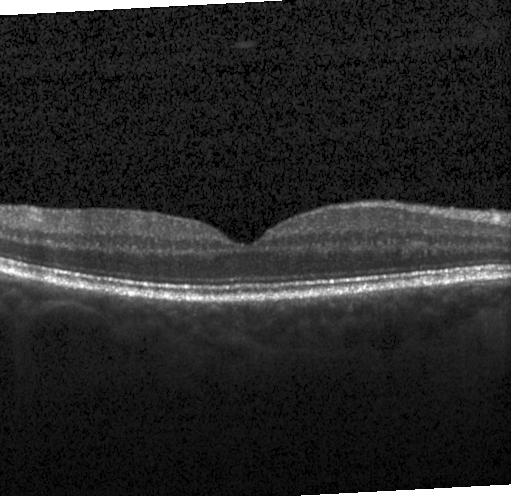 Optical coherence tomography scan.
Impression: no choroidal neovascularization, no diabetic macular edema, and no drusen.